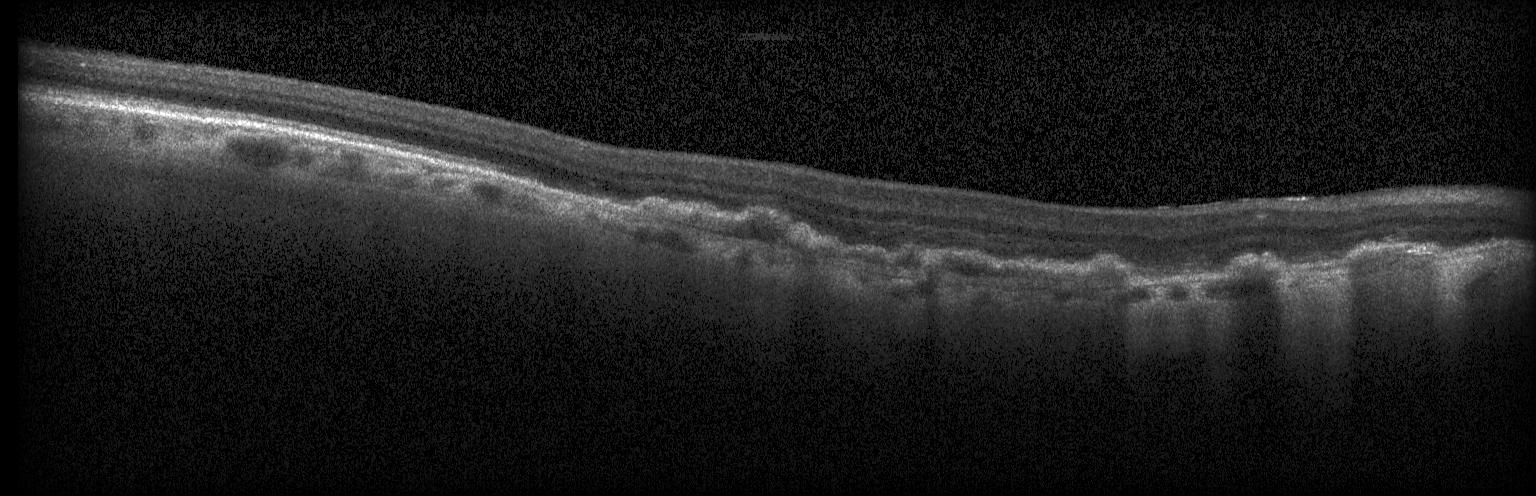

Impression: a choroidal neovascular membrane.